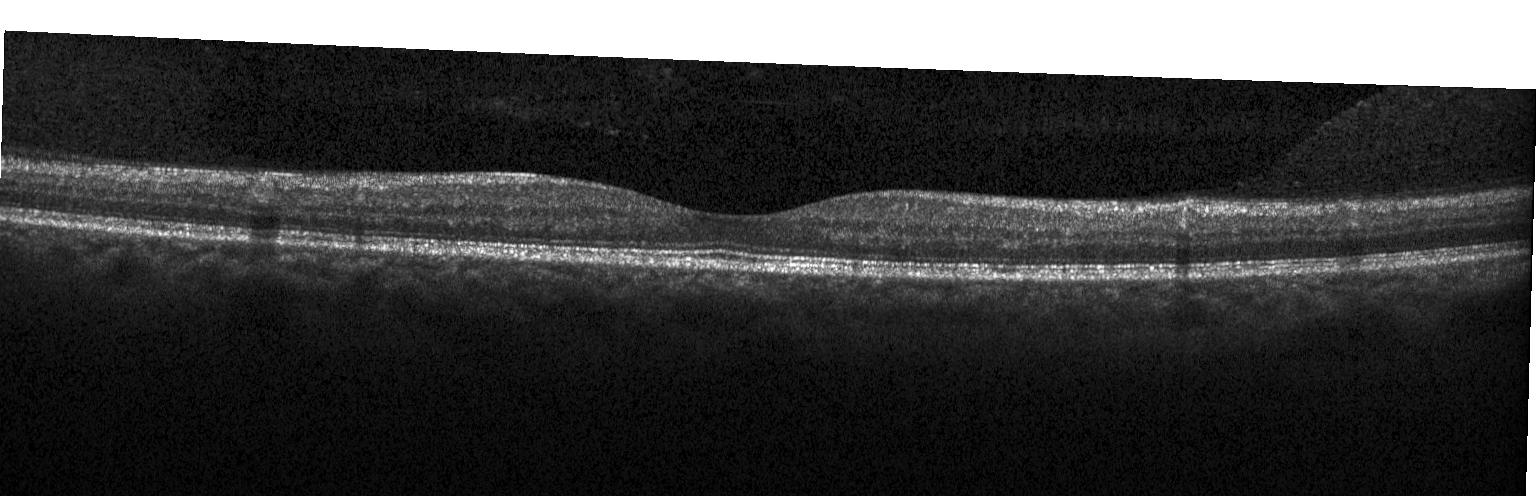 OCT line scan; macular scan; Heidelberg Spectralis OCT system; spectral-domain OCT. Diagnosis: no CNV, DME, or drusen.